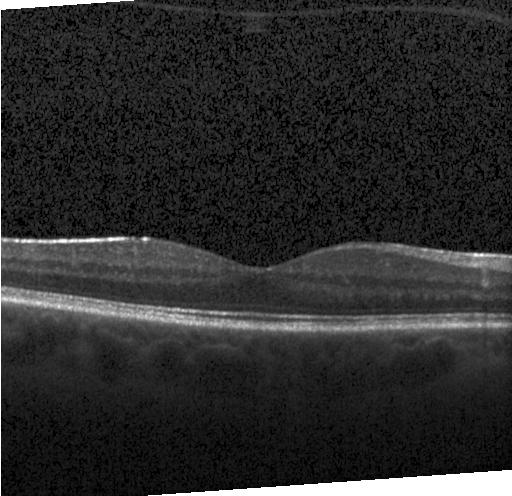

OCT scan showing neither choroidal neovascularization, diabetic macular edema, nor drusen.